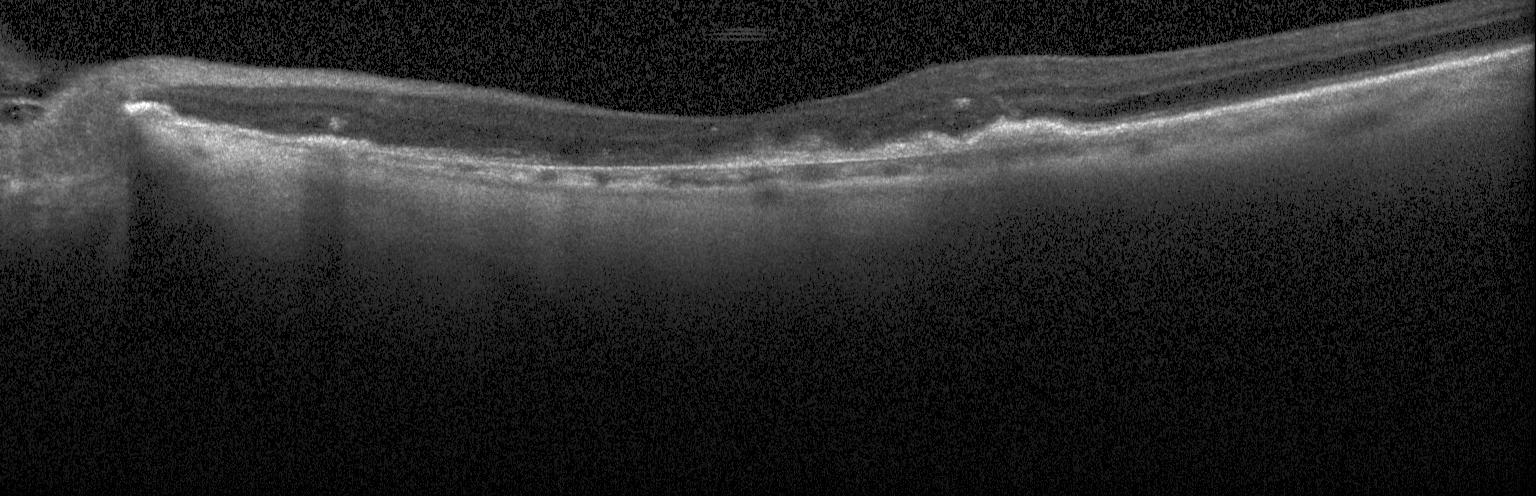

Diagnosis: choroidal neovascularization.